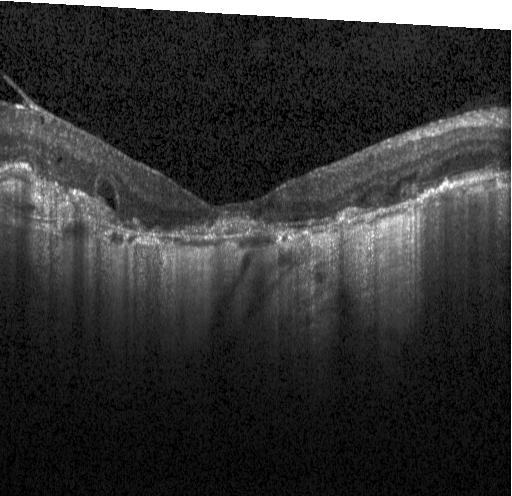
Assessment: CNV.